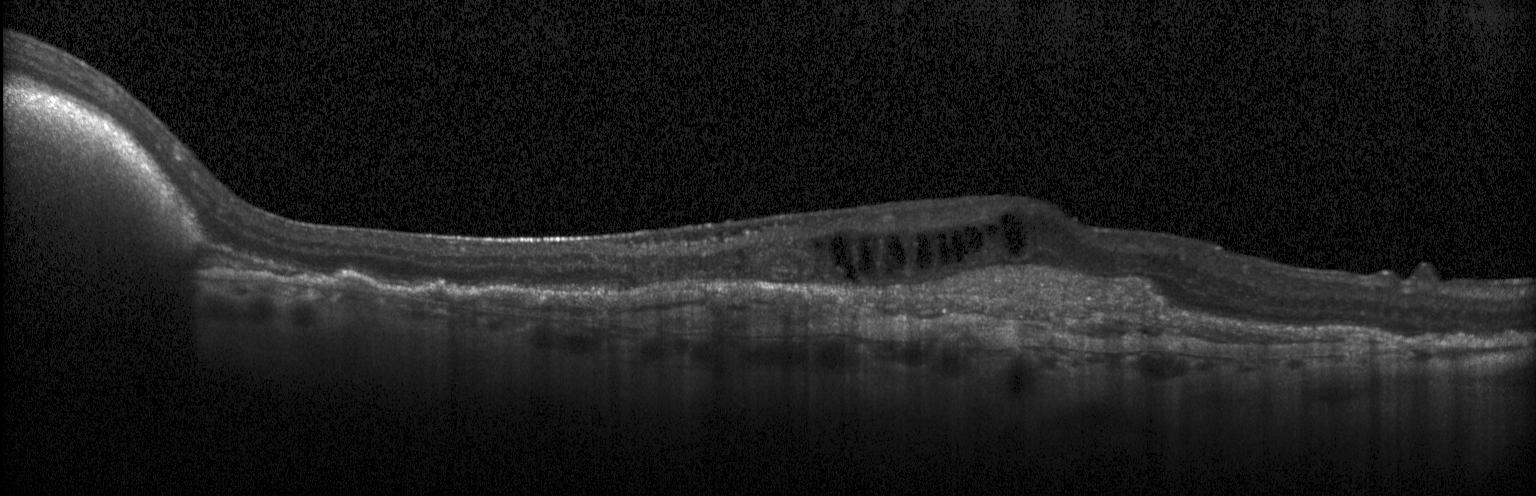

Heidelberg Spectralis OCT system; macular scan; spectral-domain OCT; OCT line scan.
Impression: a choroidal neovascular membrane.